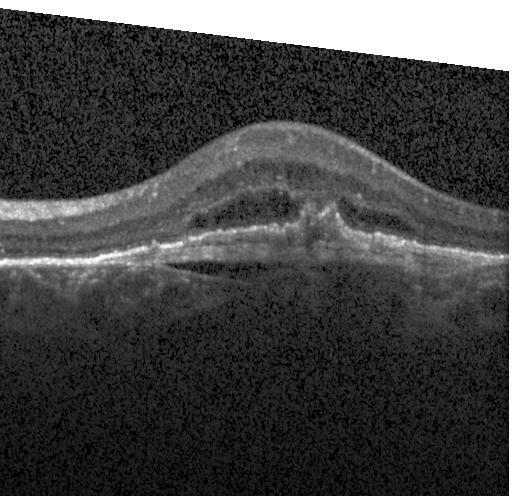 Diagnosis: CNV.